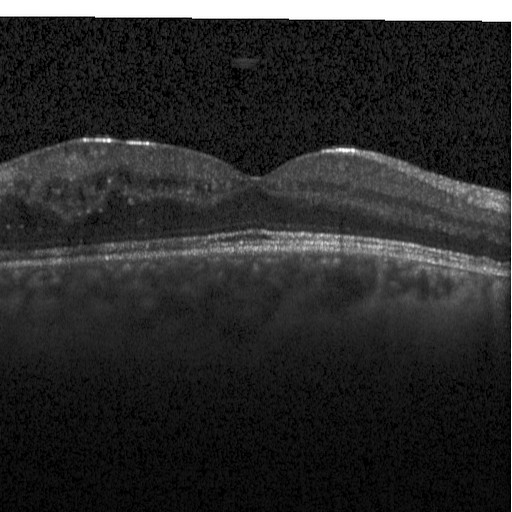
Horizontal scan through the fovea, OCT B-scan — Finding: diabetic macular edema.